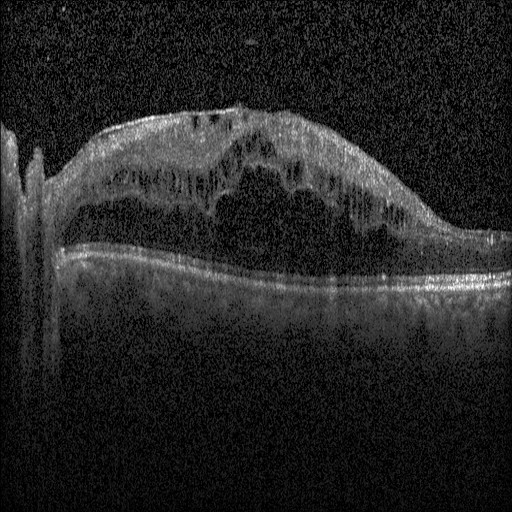 Optical coherence tomography B-scan, fovea-centered, Heidelberg Spectralis, spectral-domain optical coherence tomography.
Diabetic macular edema (DME).